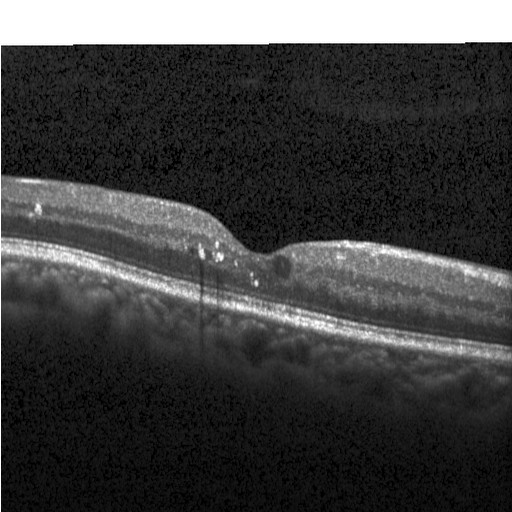 DME.